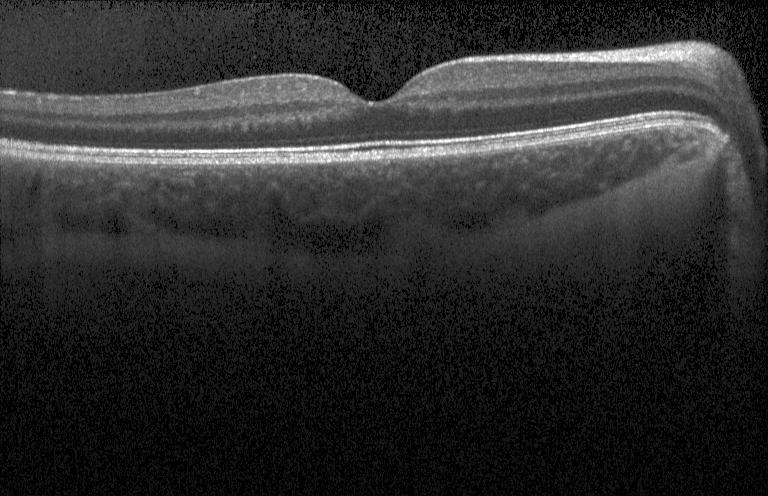

The scan shows no choroidal neovascularization, no diabetic macular edema, and no drusen.